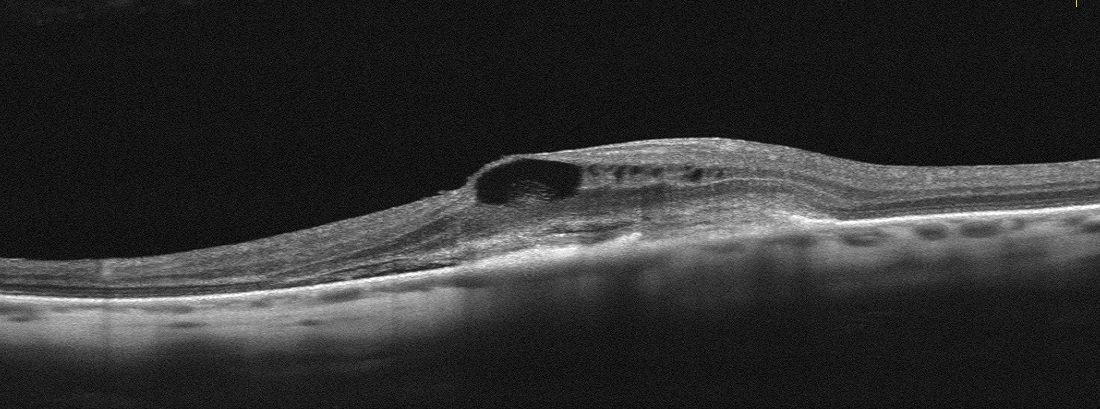

OCT B-scan · fovea-centered. This B-scan demonstrates AMD.